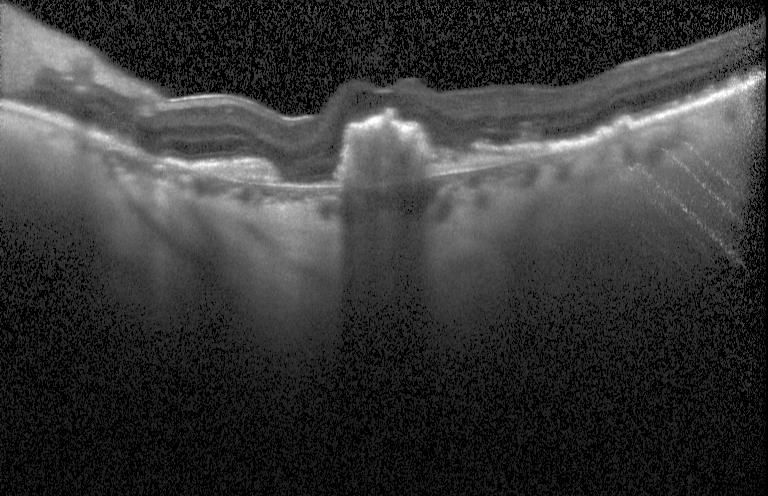
Optical coherence tomography scan, horizontal scan through the fovea, Heidelberg Spectralis OCT system — Assessment: a choroidal neovascular membrane.